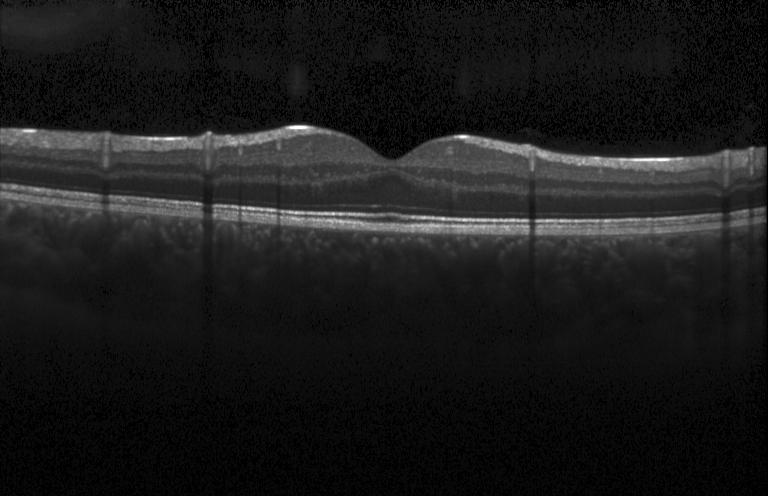 Assessment: no choroidal neovascularization, no diabetic macular edema, and no drusen.